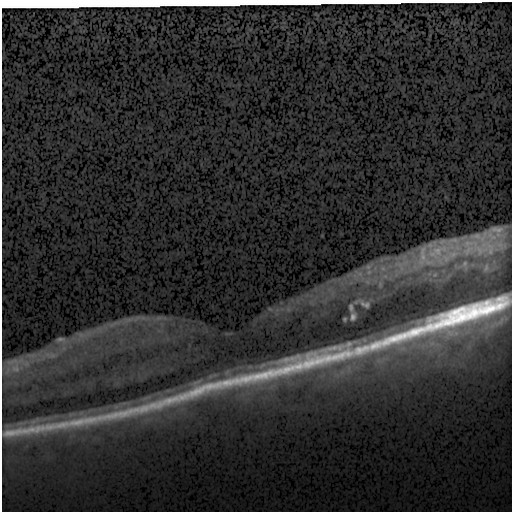 Spectral-domain optical coherence tomography. OCT line scan. Instrument: Heidelberg Spectralis
The scan shows diabetic macular edema.